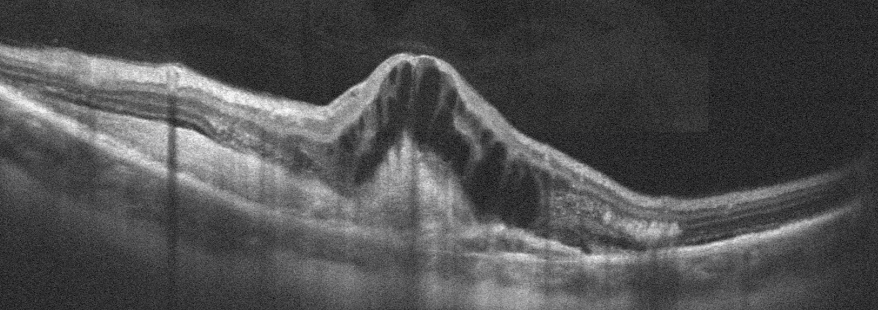
OCT finding: AMD.